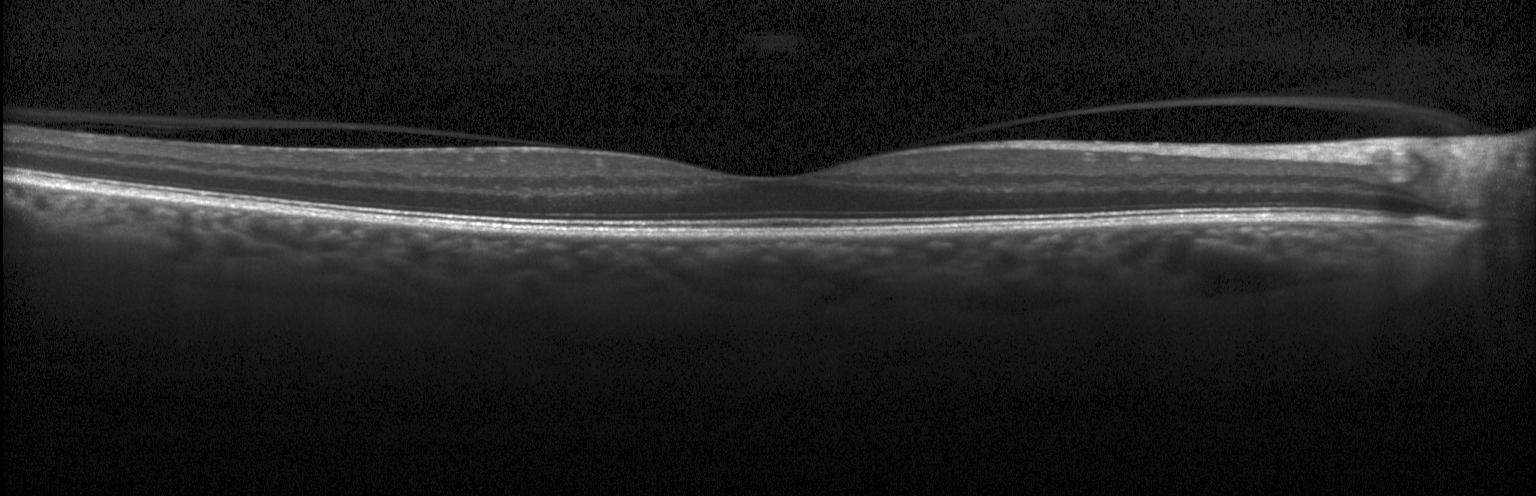 OCT finding: neither choroidal neovascularization, diabetic macular edema, nor drusen.